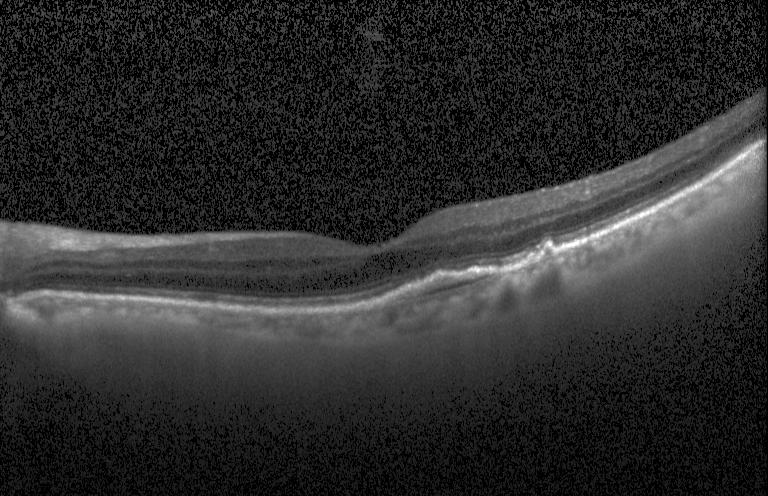 Optical coherence tomography scan.
Finding: a choroidal neovascular membrane.